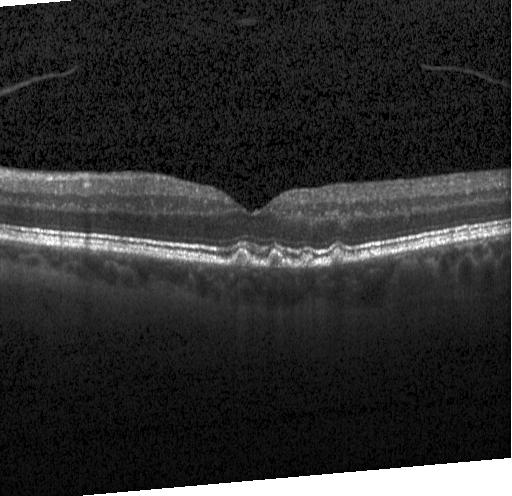

Finding: sub-RPE drusenoid deposits.